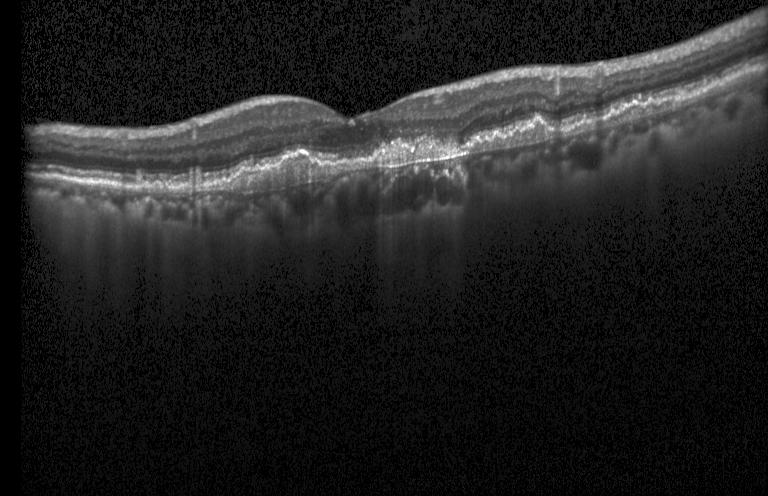

This B-scan demonstrates a choroidal neovascular membrane.